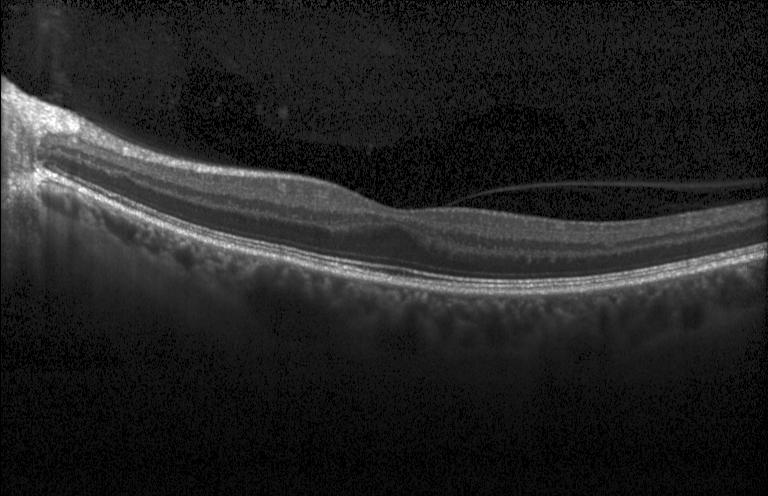

OCT line scan; fovea-centered; SD-OCT.
Dx: neither CNV, DME, nor drusen.